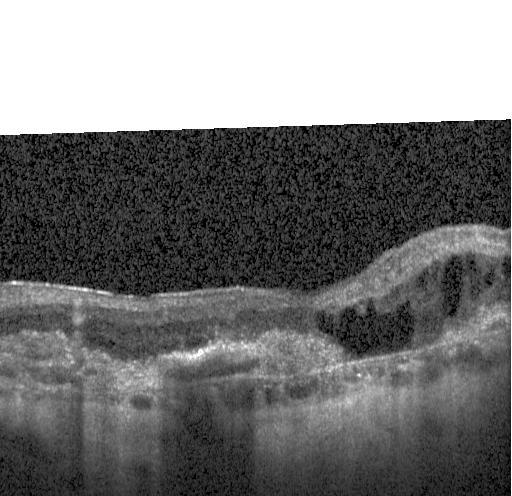 OCT line scan — This B-scan demonstrates a choroidal neovascular membrane.